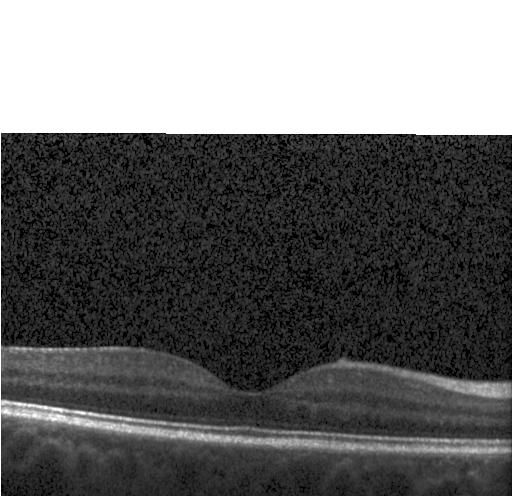
Optical coherence tomography B-scan — This B-scan demonstrates neither choroidal neovascularization, diabetic macular edema, nor drusen.